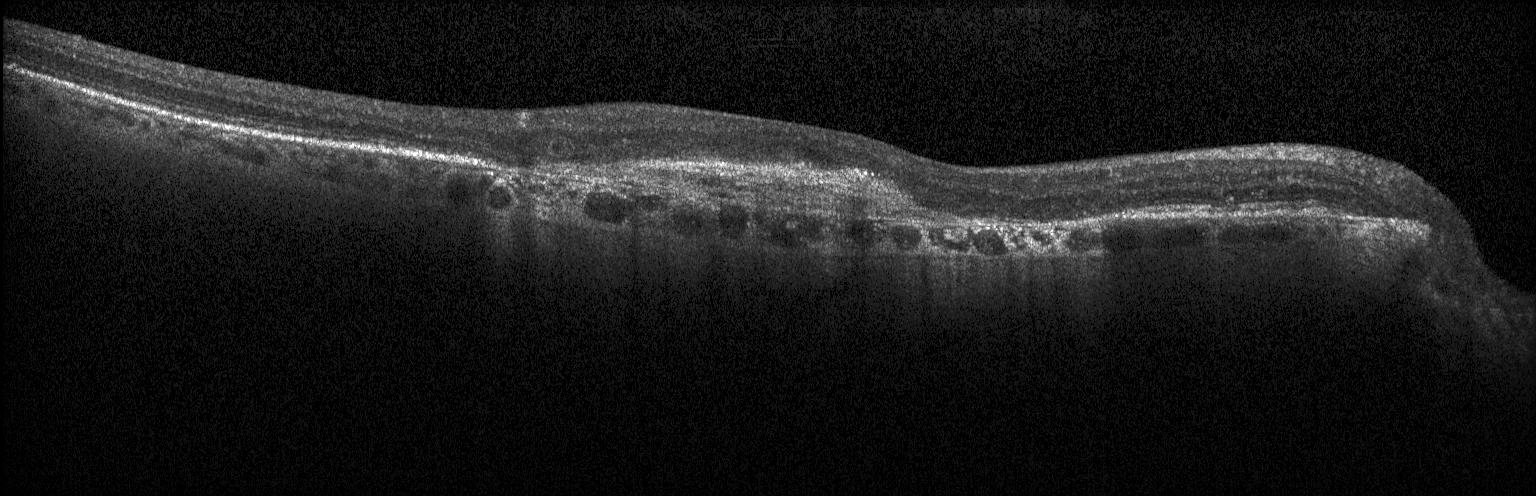

OCT line scan; spectral-domain optical coherence tomography; centered on the fovea — Choroidal neovascularization (CNV).